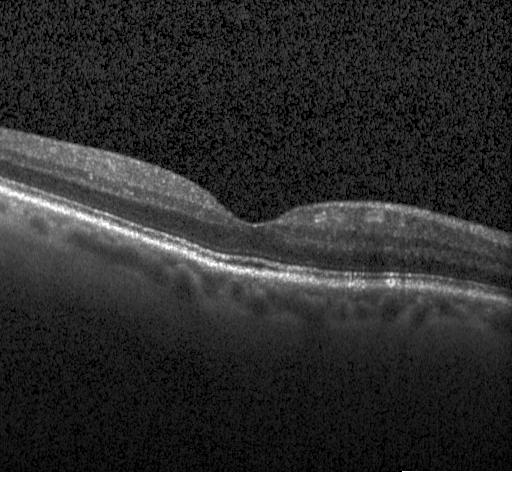
Macular OCT: no evidence of CNV, DME, or drusen.